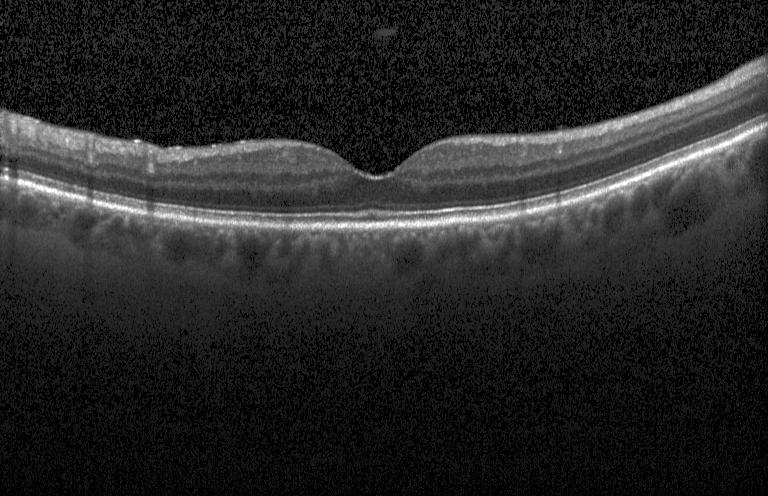

Retinal OCT B-scan. Diagnosis: neither choroidal neovascularization, diabetic macular edema, nor drusen.